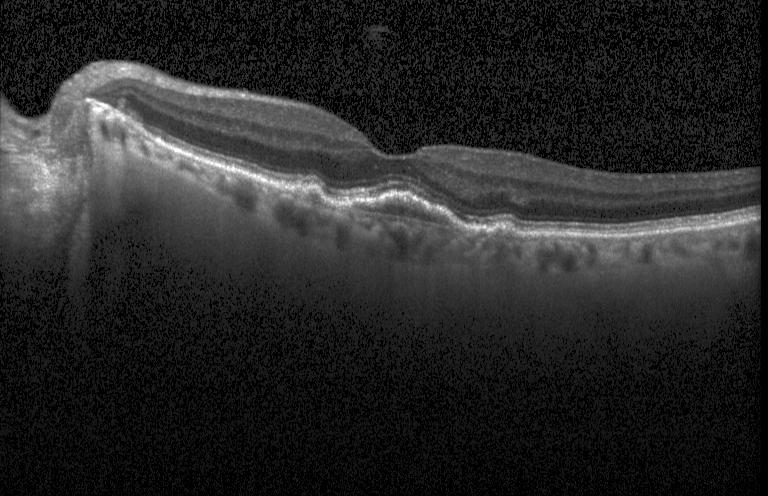 This B-scan demonstrates a choroidal neovascular membrane.